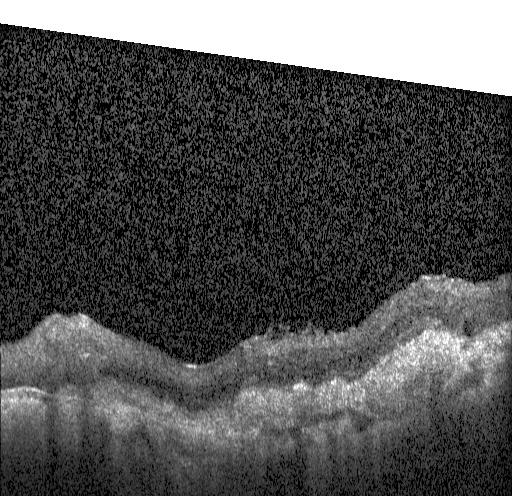
Optical coherence tomography B-scan
Impression: a choroidal neovascular membrane.